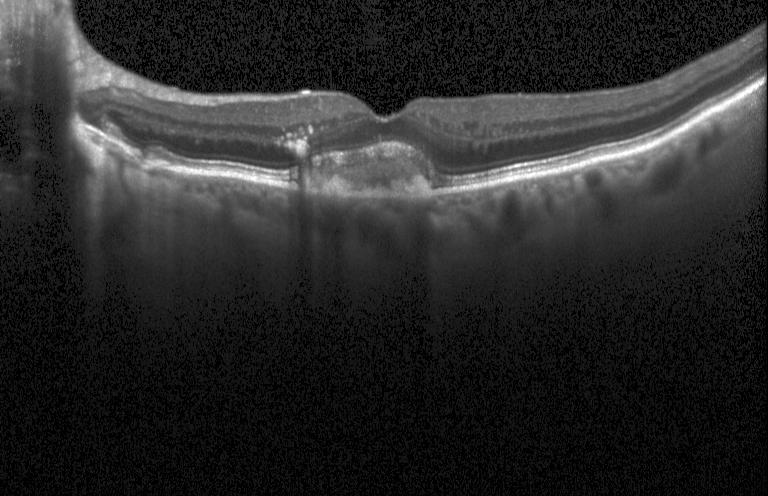

OCT line scan · Heidelberg Spectralis OCT system · SD-OCT · through the macula.
Finding: choroidal neovascularization (CNV).